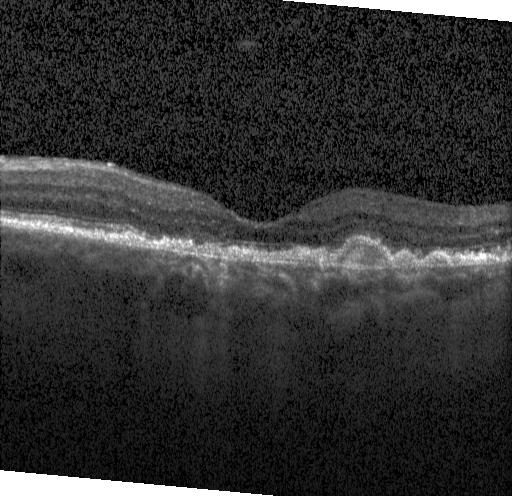

Spectral-domain optical coherence tomography; macular scan; optical coherence tomography B-scan — The scan shows a choroidal neovascular membrane.